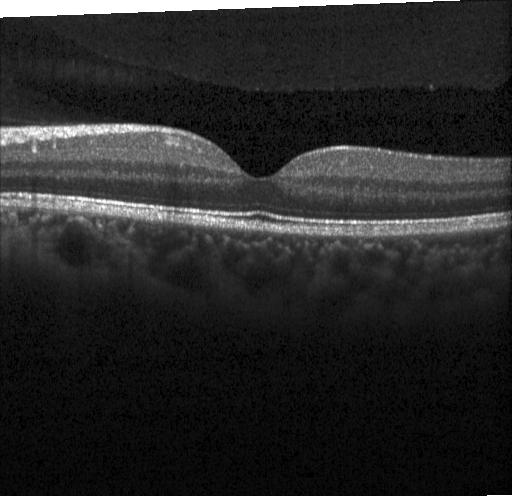
OCT B-scan showing neither CNV, DME, nor drusen.